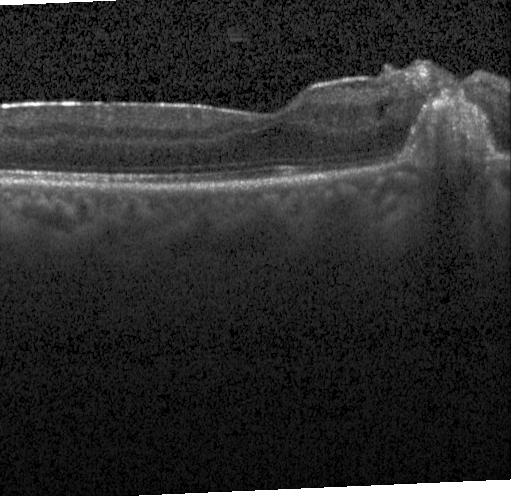
Spectral-domain OCT. Retinal OCT B-scan
OCT finding: CNV.